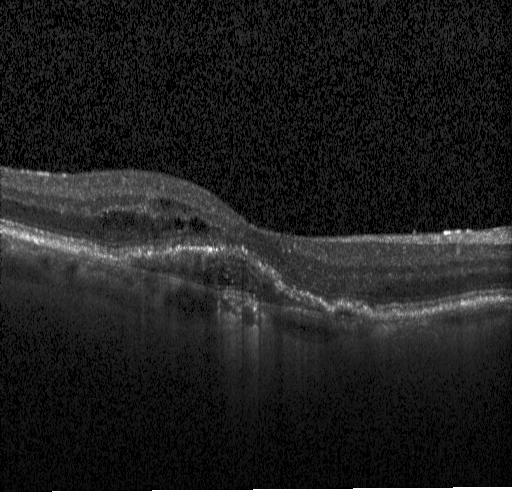
Fovea-centered · retinal OCT B-scan
Impression: CNV.